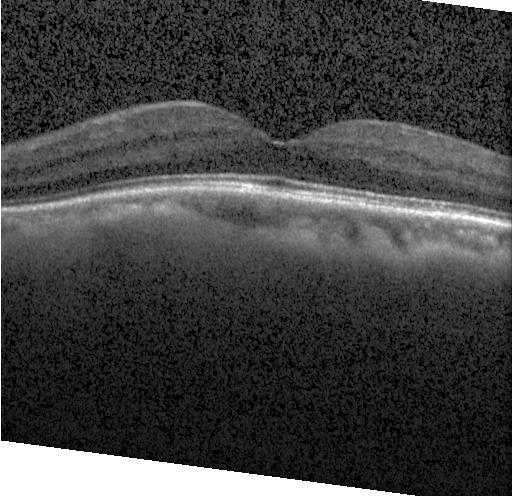
Impression: no evidence of CNV, DME, or drusen.